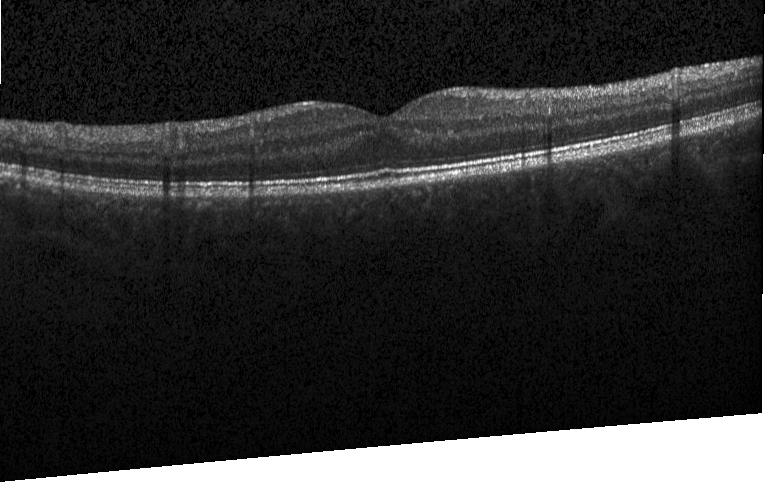
Retinal OCT B-scan, macular scan, spectral-domain optical coherence tomography, instrument: Heidelberg Spectralis. Finding: neither choroidal neovascularization, diabetic macular edema, nor drusen.